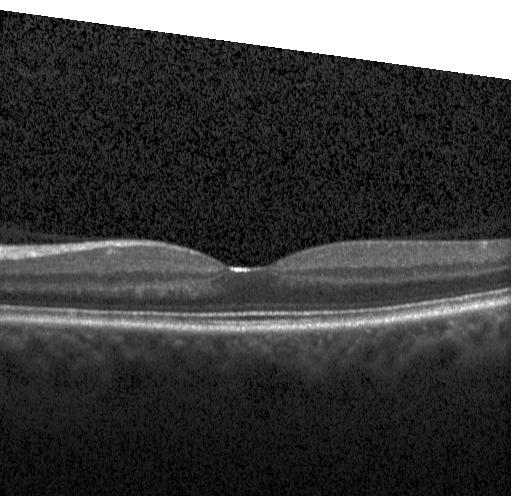

Neither choroidal neovascularization, diabetic macular edema, nor drusen.